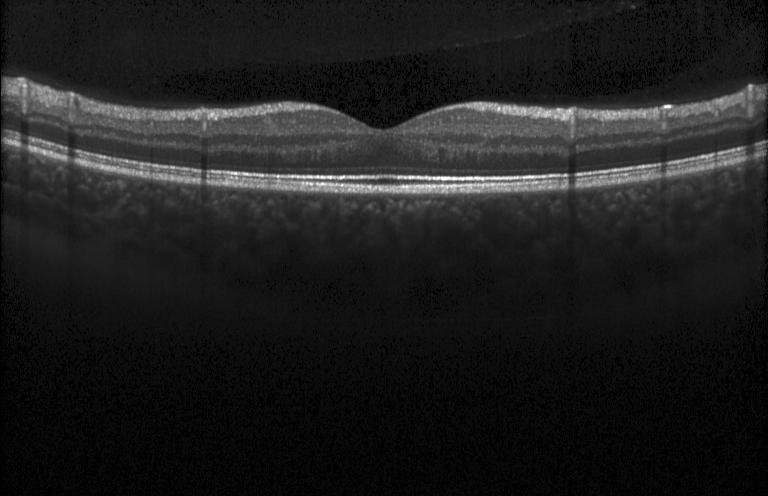 OCT B-scan; macular scan; acquired on a Heidelberg Spectralis; spectral-domain optical coherence tomography.
This B-scan demonstrates neither choroidal neovascularization, diabetic macular edema, nor drusen.